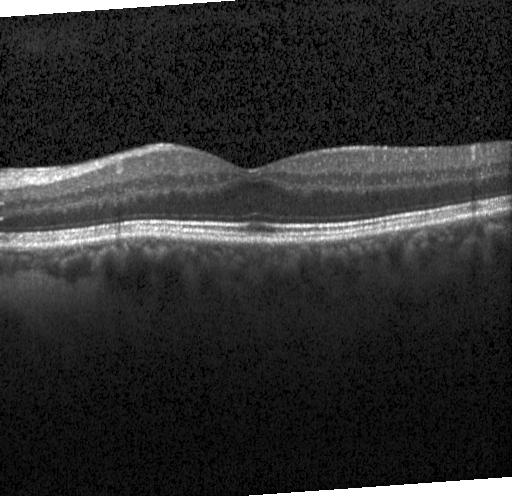 OCT finding: no choroidal neovascularization, diabetic macular edema, or drusen.